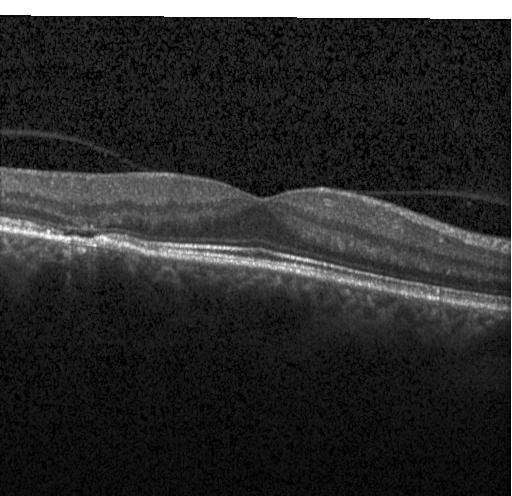
Retinal OCT B-scan — A choroidal neovascular membrane.